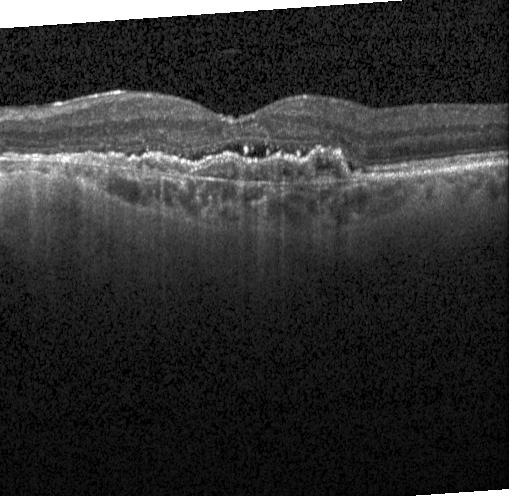 OCT scan showing a choroidal neovascular membrane.